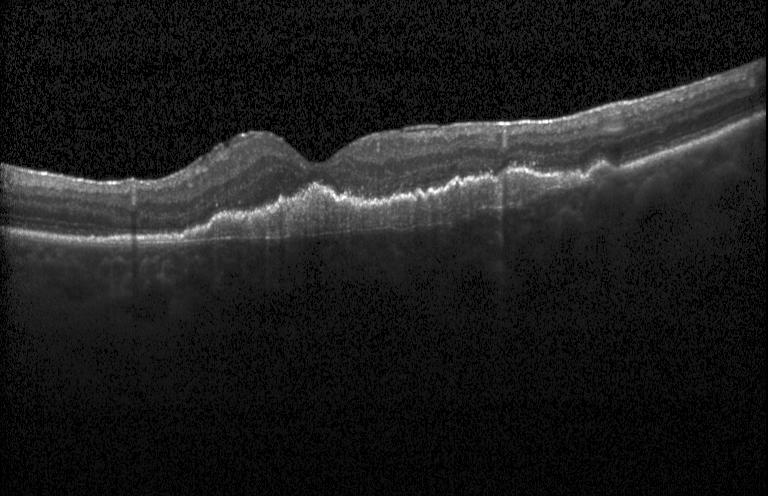
Acquired on a Heidelberg Spectralis; OCT line scan; through the macula; SD-OCT.
Finding: a choroidal neovascular membrane.